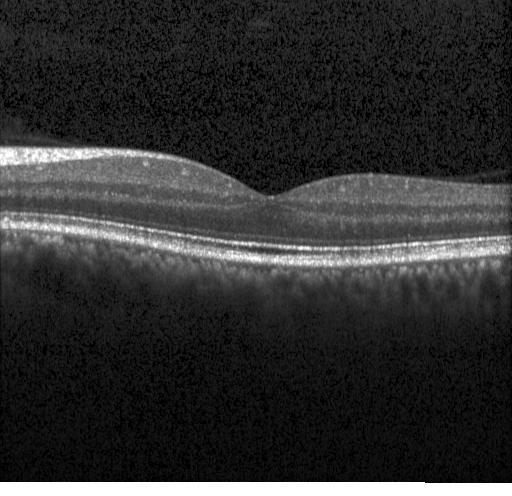 OCT line scan.
The scan shows neither choroidal neovascularization, diabetic macular edema, nor drusen.